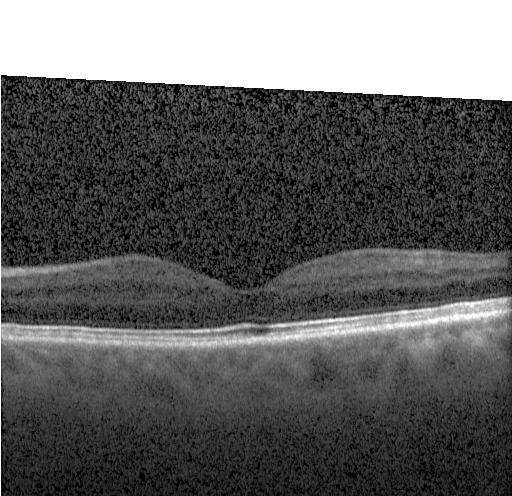 Spectral-domain OCT; OCT line scan; instrument: Heidelberg Spectralis; centered on the fovea.
Diagnosis: neither choroidal neovascularization, diabetic macular edema, nor drusen.